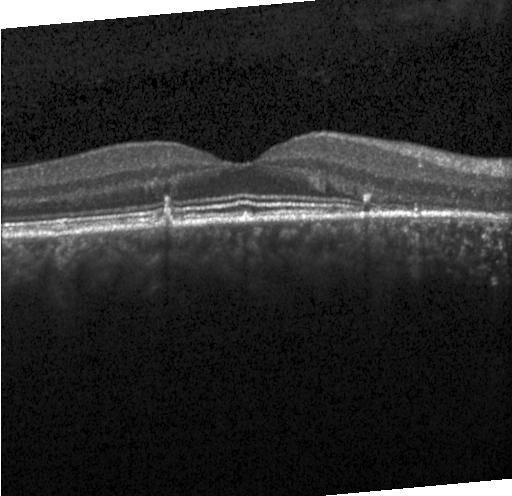

Macular scan; optical coherence tomography scan. Diagnosis: sub-RPE drusenoid deposits.